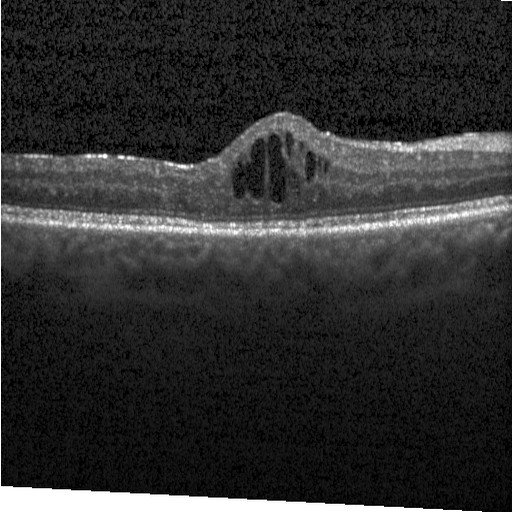 OCT B-scan. Spectral-domain OCT.
OCT finding: diabetic macular edema (DME).